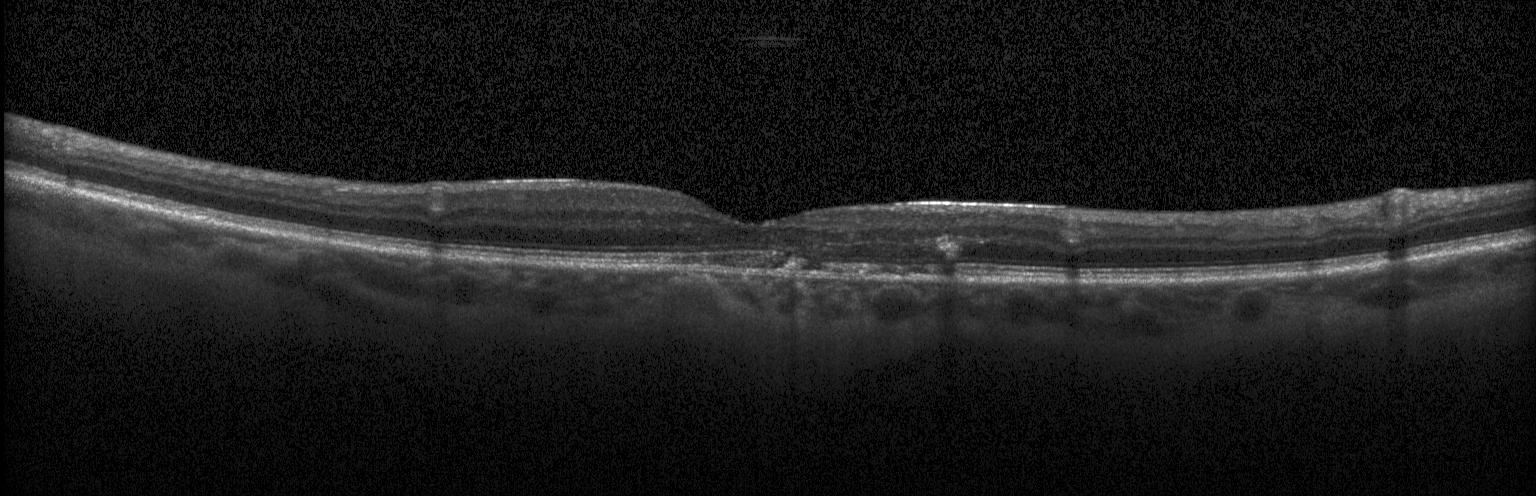 OCT B-scan. Finding: choroidal neovascularization (CNV).